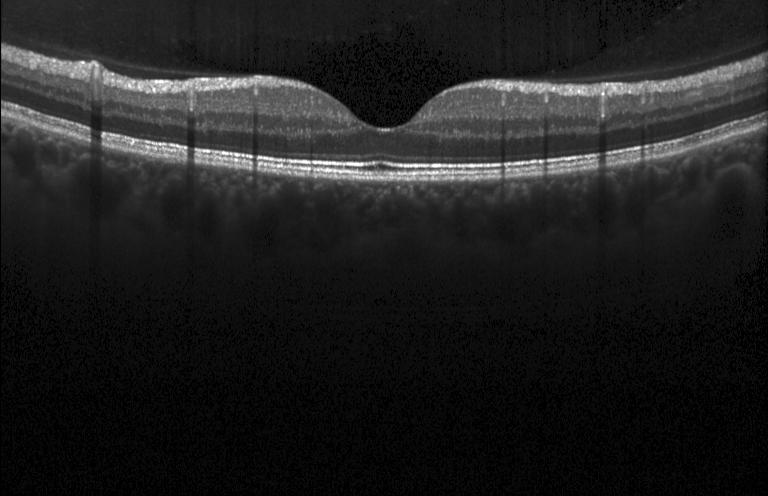 Acquired on a Heidelberg Spectralis; OCT line scan; spectral-domain optical coherence tomography; horizontal scan through the fovea. The scan shows neither choroidal neovascularization, diabetic macular edema, nor drusen.